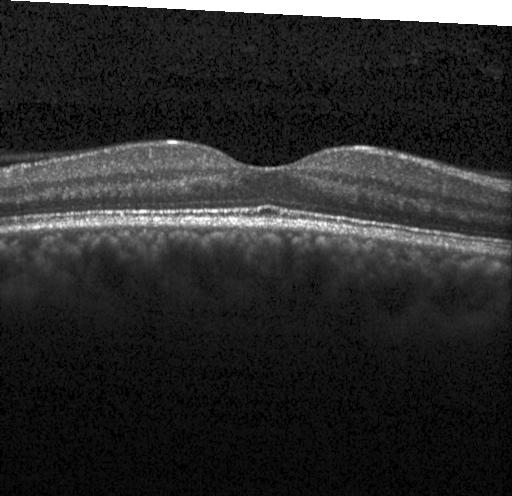

Optical coherence tomography B-scan. Impression: no evidence of choroidal neovascularization, diabetic macular edema, or drusen.